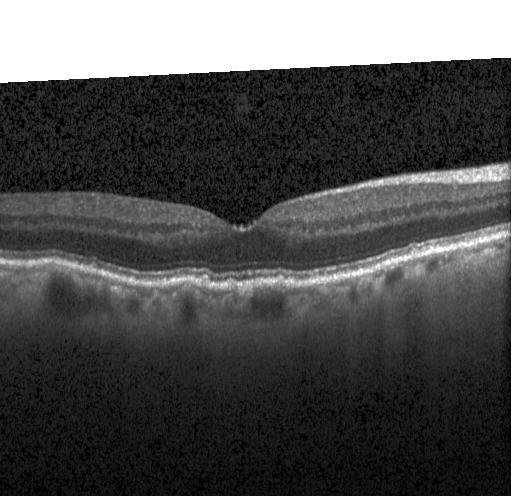 Heidelberg Spectralis OCT system; OCT line scan; spectral-domain OCT
Finding: sub-RPE drusenoid deposits.